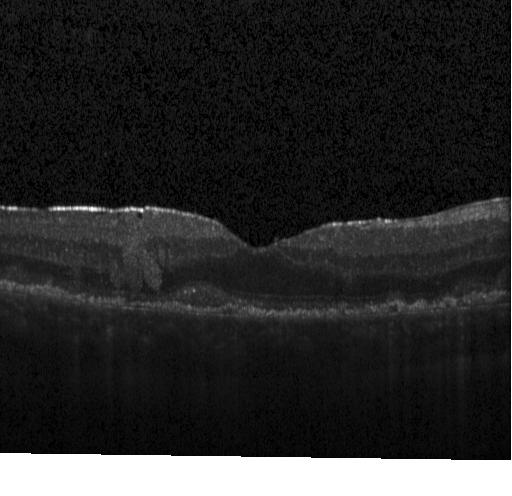

Heidelberg Spectralis. SD-OCT. Optical coherence tomography B-scan.
This B-scan demonstrates a choroidal neovascular membrane.